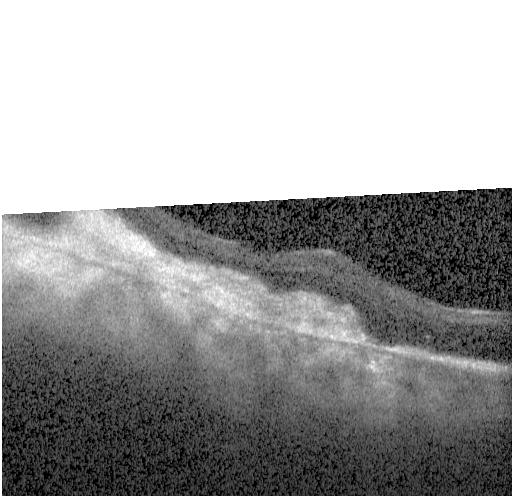

The scan shows choroidal neovascularization.